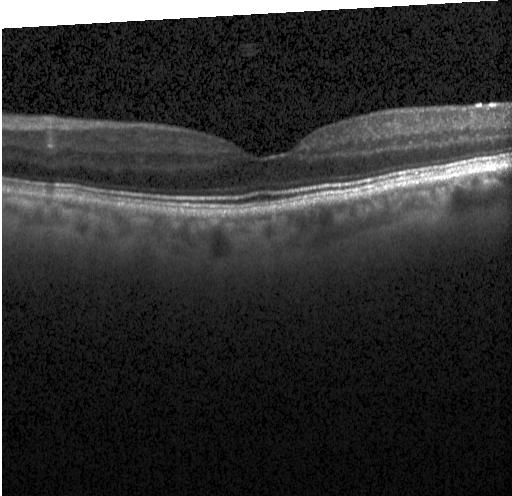

Dx: no evidence of choroidal neovascularization, diabetic macular edema, or drusen.